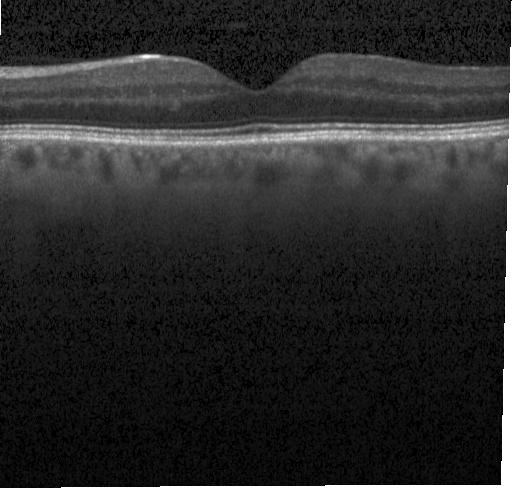
Optical coherence tomography B-scan — Finding: no CNV, DME, or drusen.